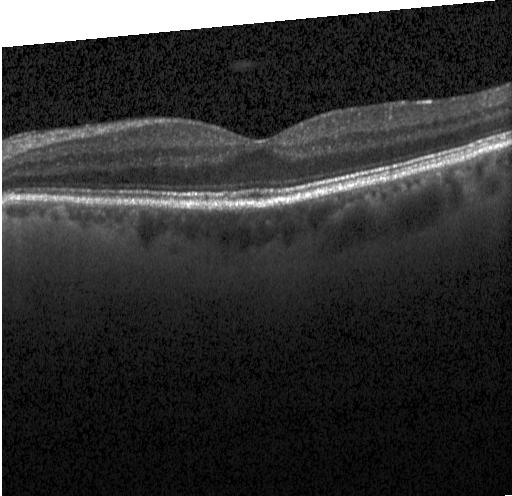 Finding: no choroidal neovascularization, diabetic macular edema, or drusen.